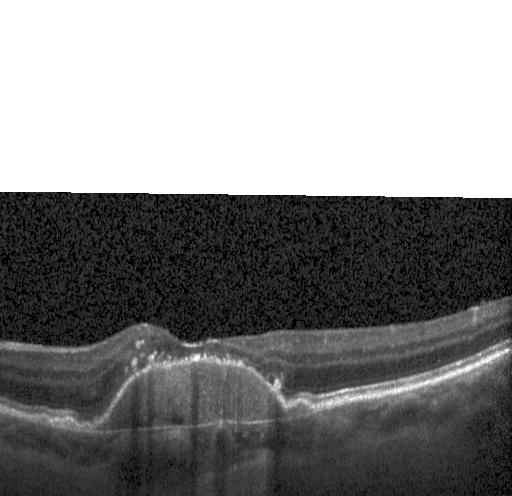
The scan shows choroidal neovascularization (CNV).